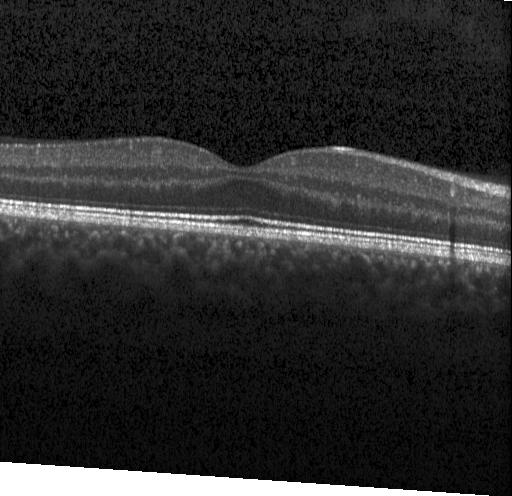

The scan shows no CNV, DME, or drusen.